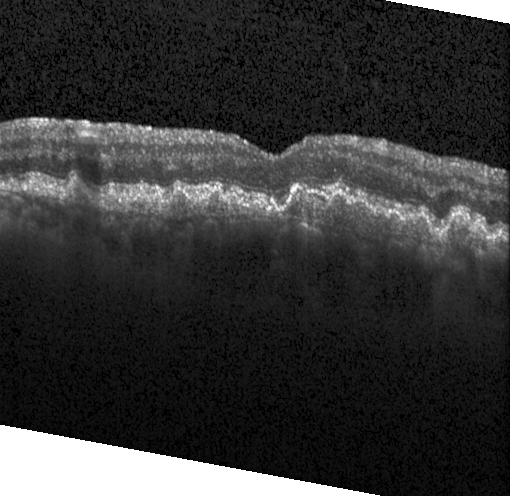
Heidelberg Spectralis OCT system, centered on the fovea, SD-OCT, optical coherence tomography scan. Impression: a choroidal neovascular membrane.